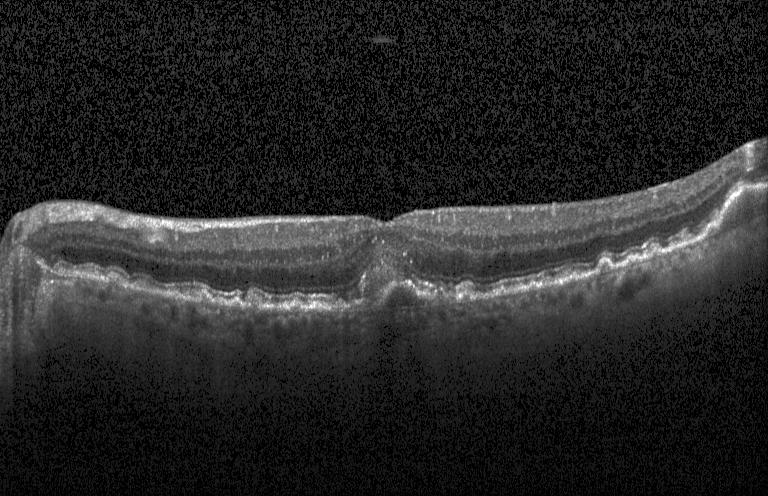

OCT line scan — OCT finding: choroidal neovascularization (CNV).